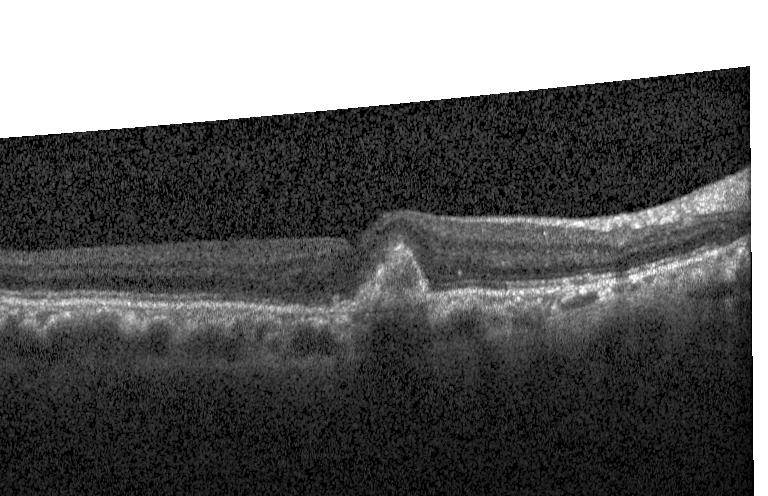

Finding: choroidal neovascularization.